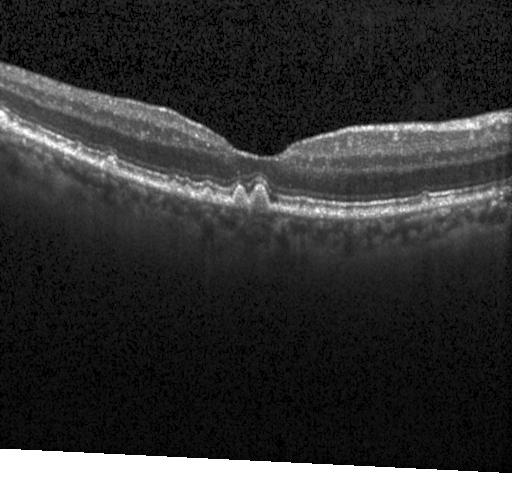 Impression: sub-RPE drusenoid deposits.